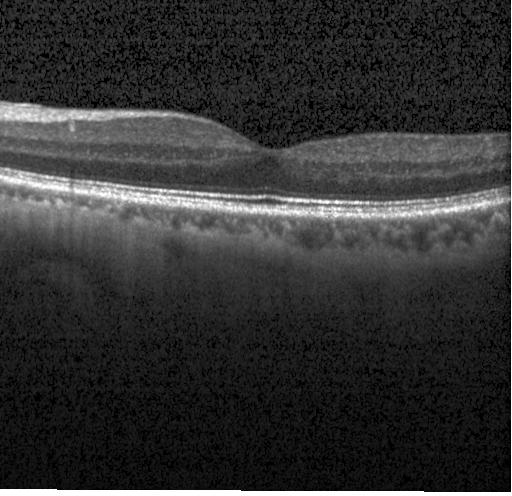
Acquired on a Heidelberg Spectralis; optical coherence tomography B-scan; fovea-centered; spectral-domain OCT.
Diagnosis: no evidence of choroidal neovascularization, diabetic macular edema, or drusen.